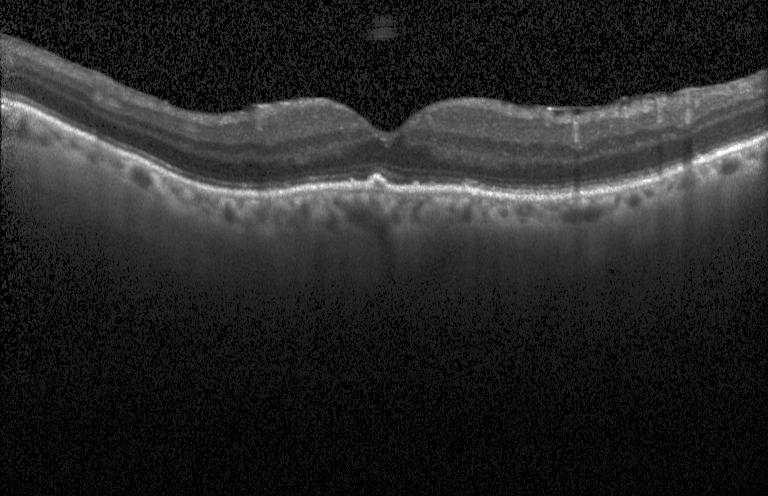

OCT finding: drusen.